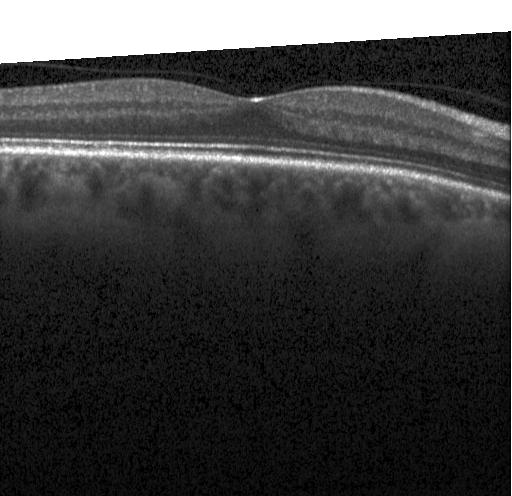

SD-OCT, OCT line scan, Heidelberg Spectralis. The scan shows no evidence of choroidal neovascularization, diabetic macular edema, or drusen.